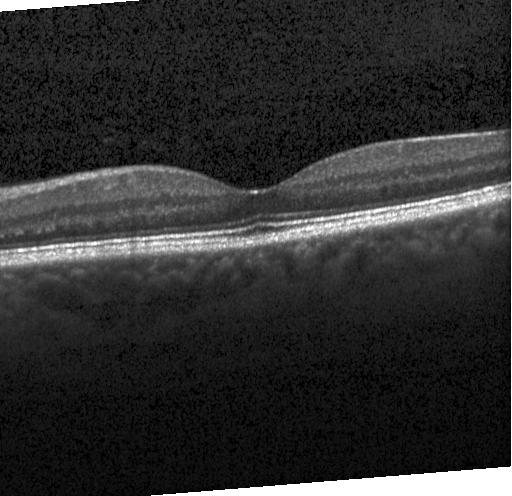
OCT line scan · Heidelberg Spectralis OCT system · SD-OCT
The scan shows no choroidal neovascularization, no diabetic macular edema, and no drusen.